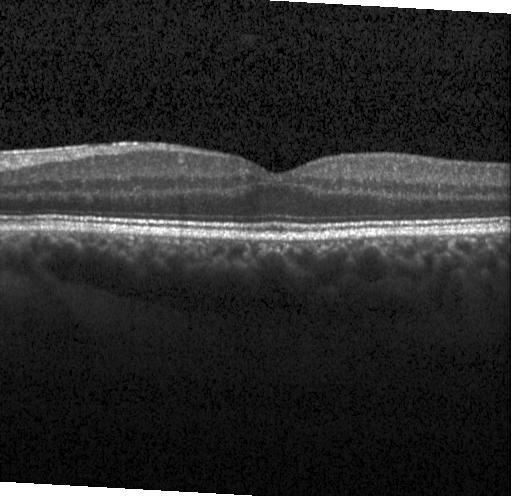
Finding: no choroidal neovascularization, no diabetic macular edema, and no drusen.